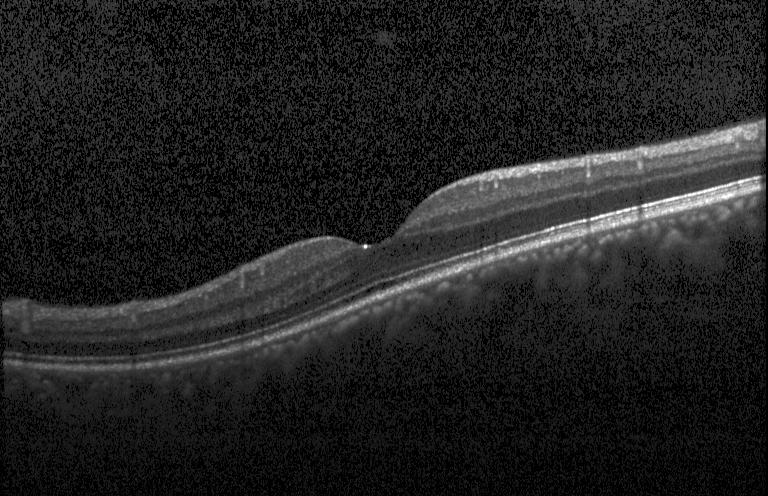 Retinal OCT cross-section showing no evidence of choroidal neovascularization, diabetic macular edema, or drusen.